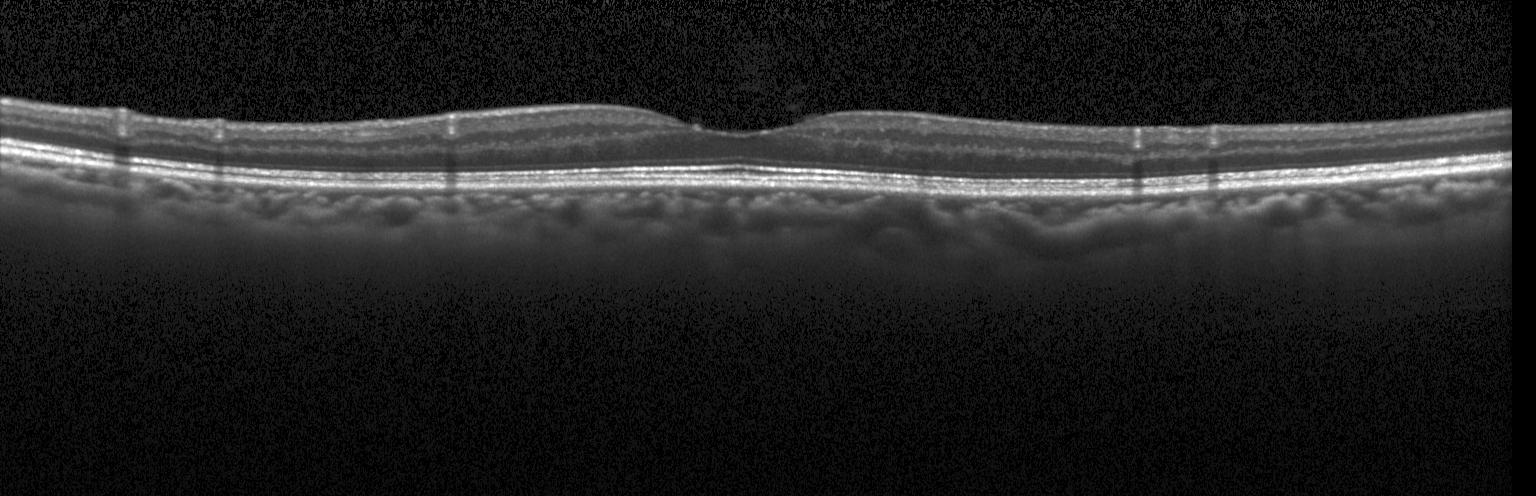

Acquired on a Heidelberg Spectralis, OCT line scan, through the macula.
Dx: no evidence of CNV, DME, or drusen.